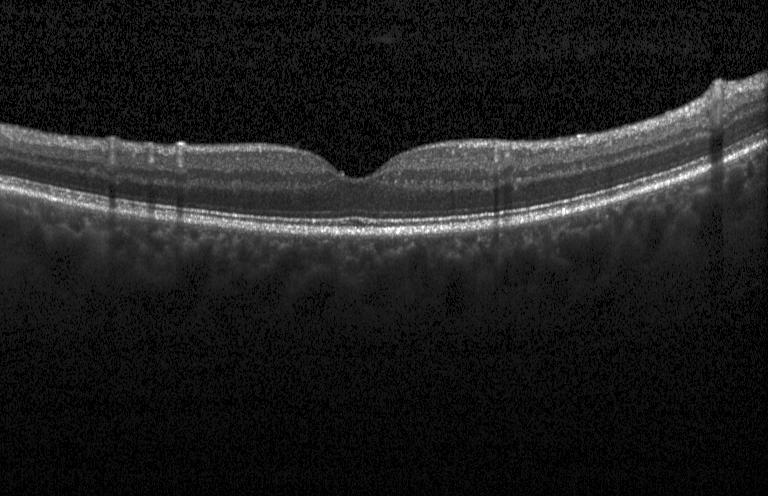

The scan shows neither choroidal neovascularization, diabetic macular edema, nor drusen.